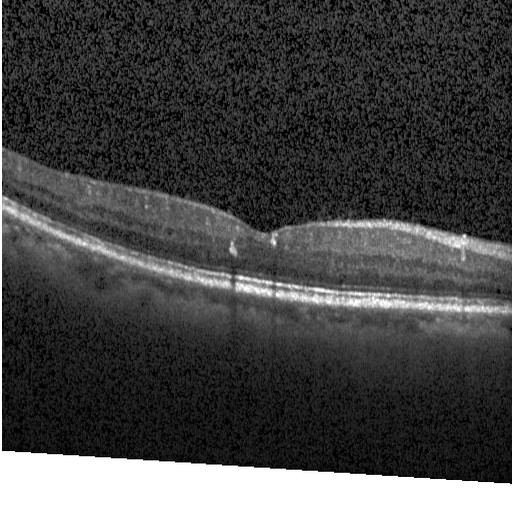
Macular OCT: DME.